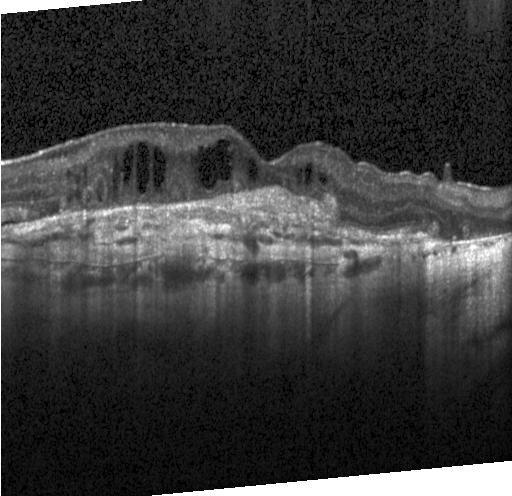 Diagnosis: choroidal neovascularization.